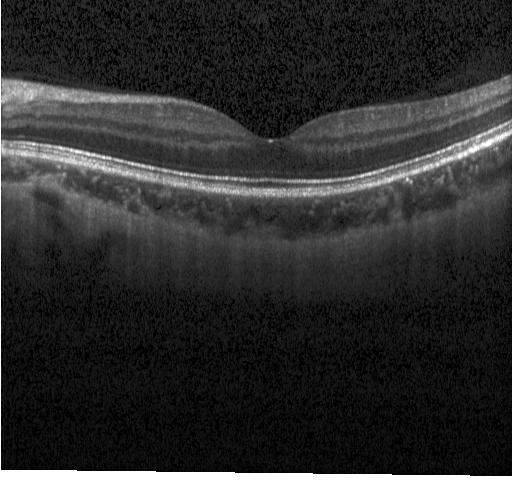

No CNV, no DME, and no drusen.